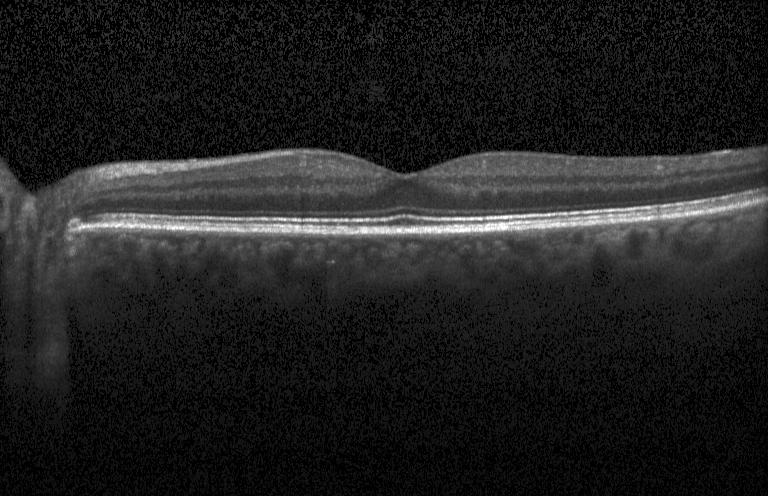

OCT B-scan. Impression: no CNV, no DME, and no drusen.